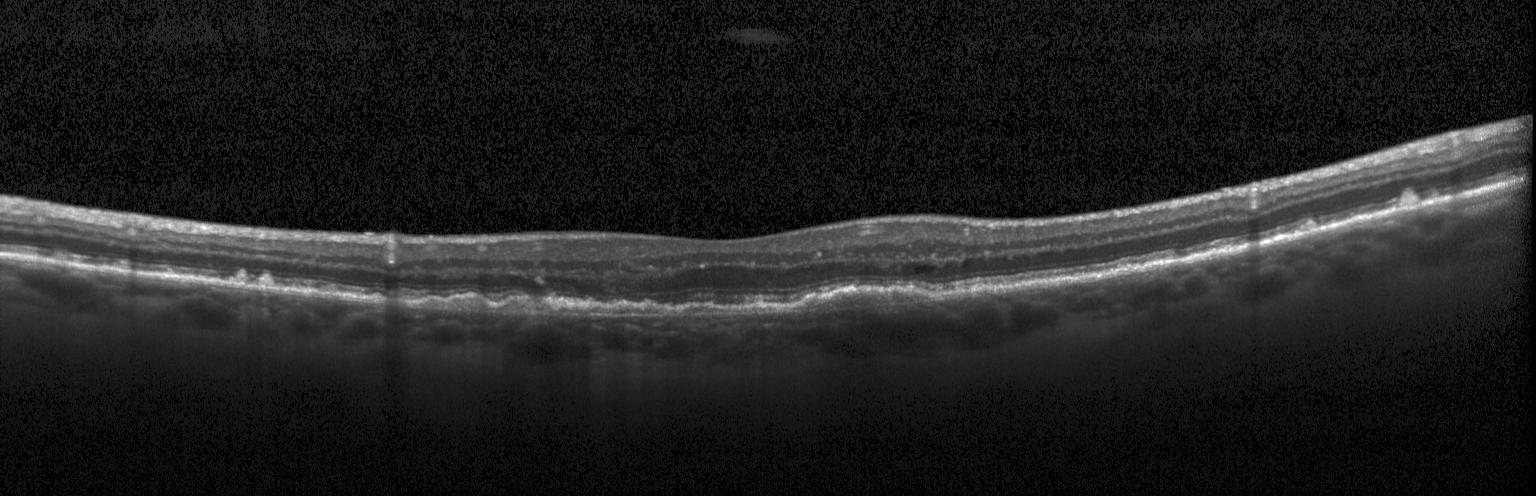 OCT line scan
Assessment: choroidal neovascularization (CNV).